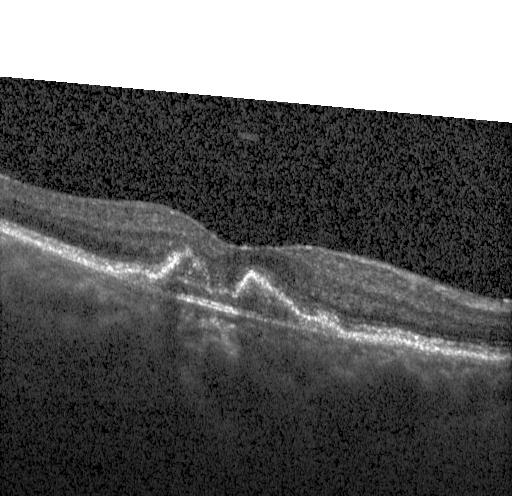
Assessment: a choroidal neovascular membrane.